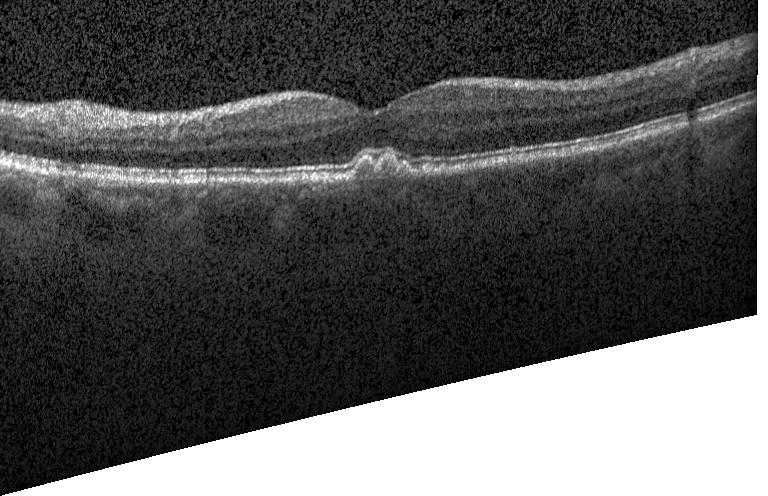

Retinal OCT B-scan — Impression: multiple drusen.